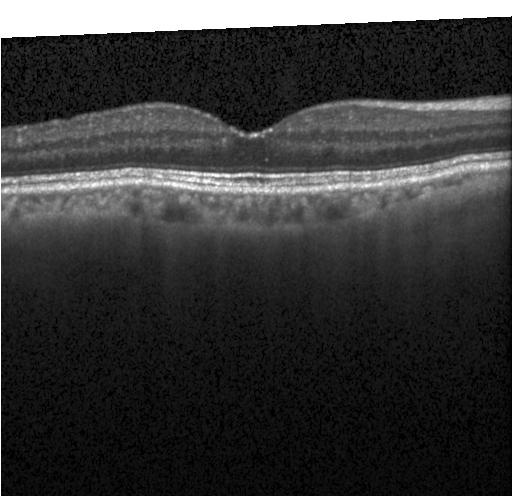

Optical coherence tomography scan · instrument: Heidelberg Spectralis
Diagnosis: no evidence of CNV, DME, or drusen.